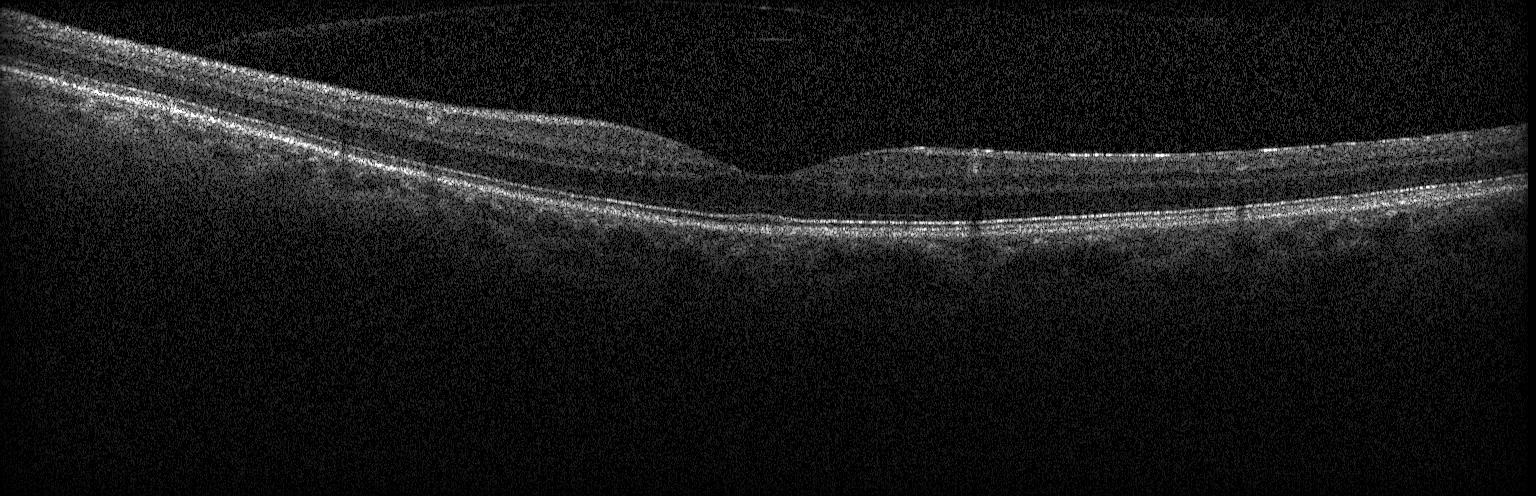

Spectral-domain OCT, macular scan, acquired on a Heidelberg Spectralis, retinal OCT cross-section
The scan shows neither choroidal neovascularization, diabetic macular edema, nor drusen.